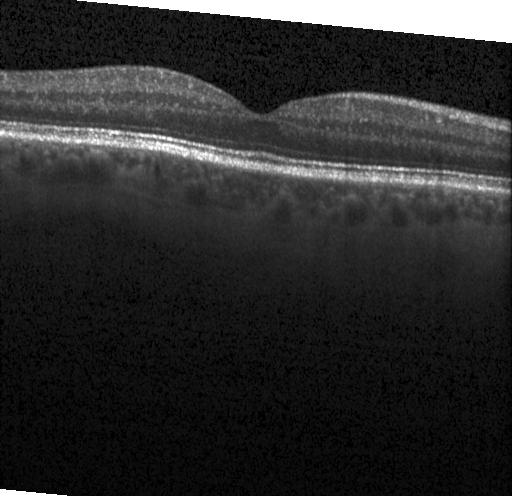

Diagnosis: neither choroidal neovascularization, diabetic macular edema, nor drusen.